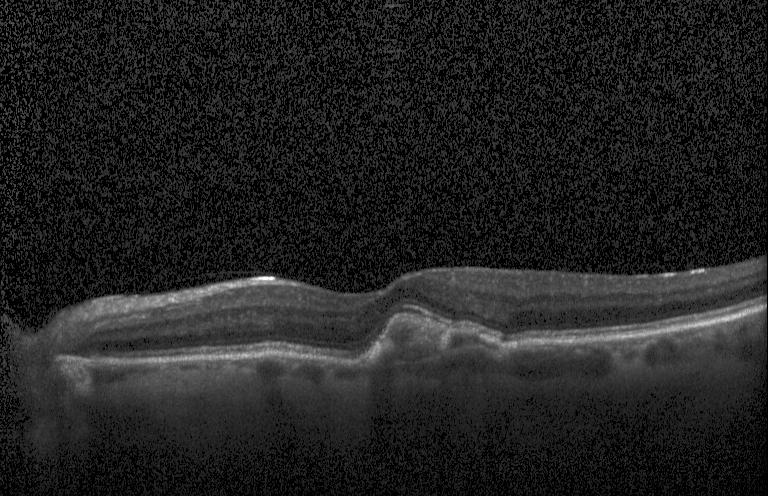 Optical coherence tomography scan. SD-OCT. Heidelberg Spectralis. Fovea-centered
Finding: a choroidal neovascular membrane.